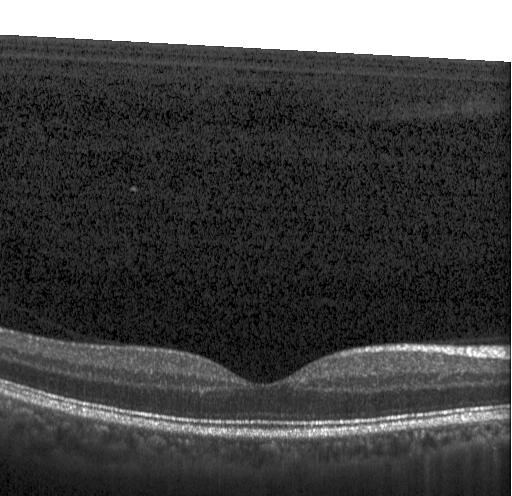 Acquired on a Heidelberg Spectralis. SD-OCT. Horizontal scan through the fovea. Retinal OCT B-scan.
This B-scan demonstrates neither CNV, DME, nor drusen.